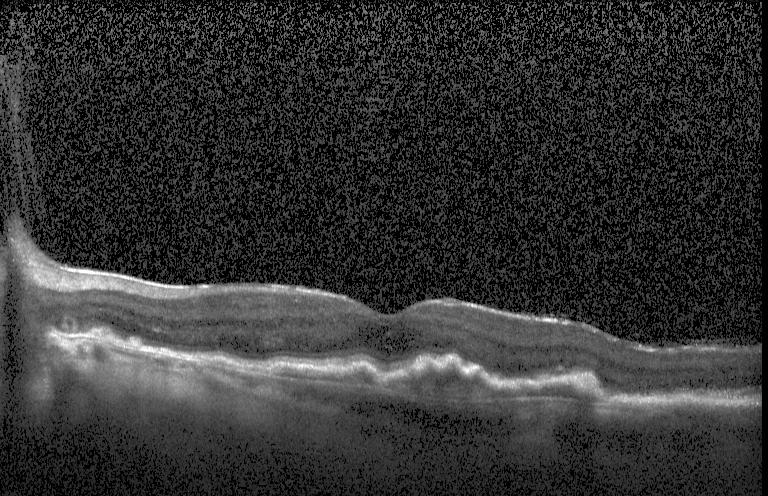
This B-scan demonstrates a choroidal neovascular membrane.